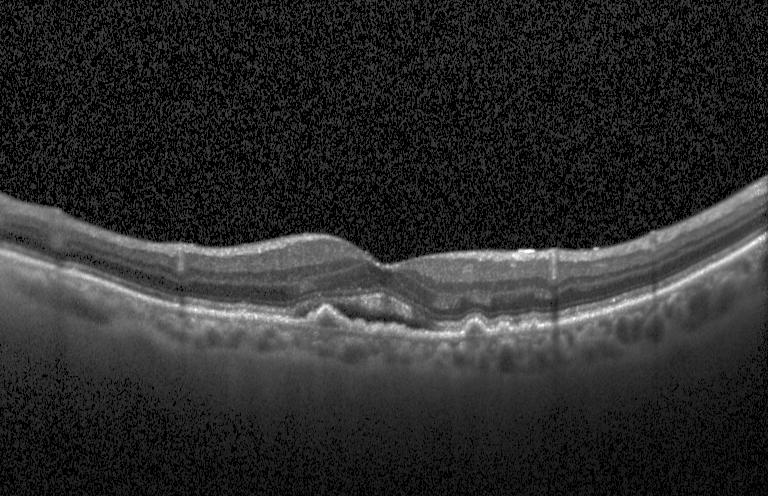
The scan shows a choroidal neovascular membrane.